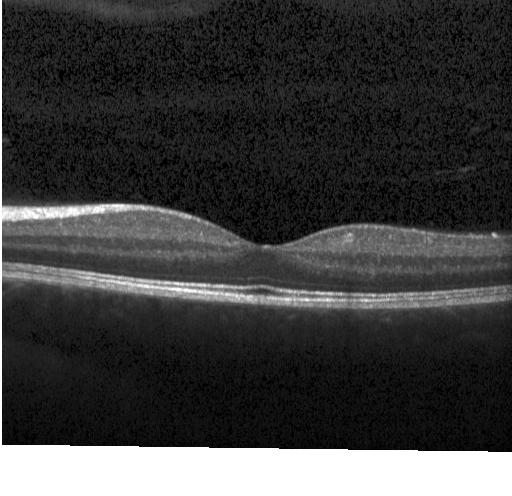
Optical coherence tomography B-scan.
The scan shows no CNV, no DME, and no drusen.